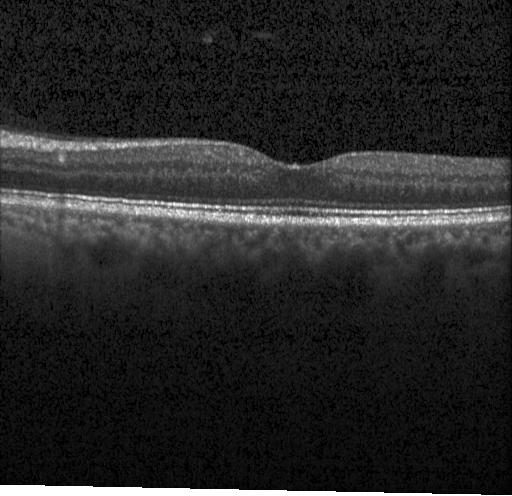

Retinal OCT cross-section showing no evidence of choroidal neovascularization, diabetic macular edema, or drusen.